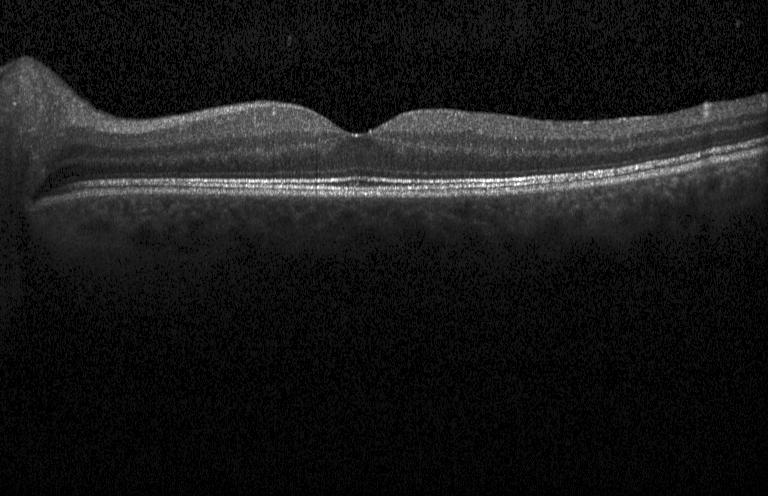 Retinal OCT B-scan.
No CNV, DME, or drusen.